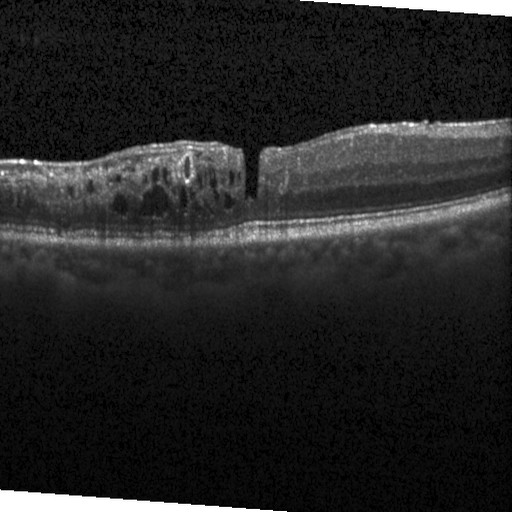

Finding: DME.